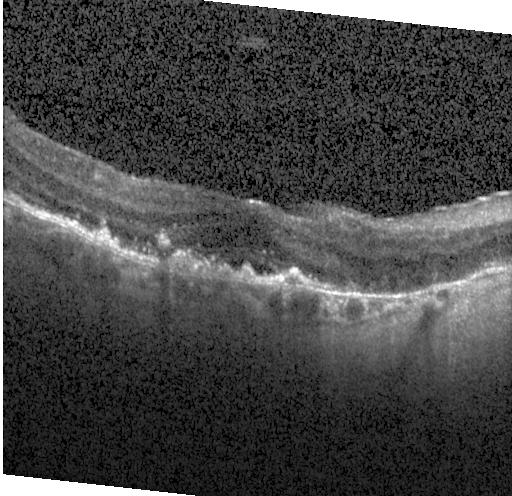

Acquired on a Heidelberg Spectralis; horizontal scan through the fovea; OCT B-scan.
Diagnosis: a choroidal neovascular membrane.